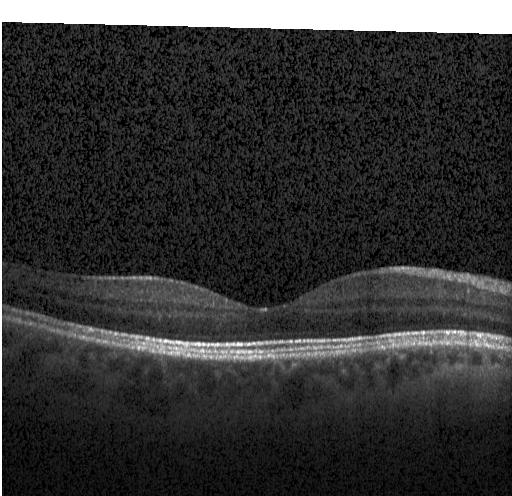
Retinal OCT cross-section. Neither CNV, DME, nor drusen.